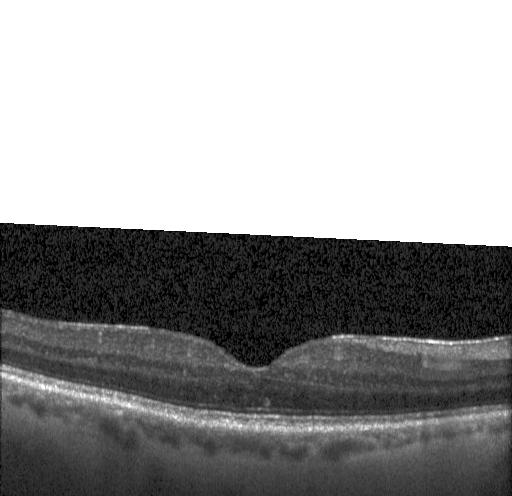

OCT scan showing no choroidal neovascularization, diabetic macular edema, or drusen.